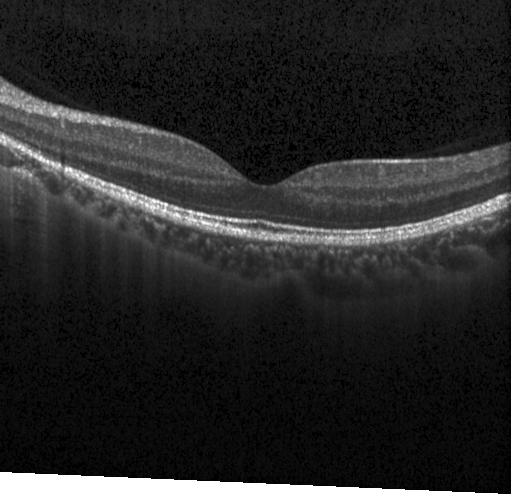 Diagnosis: no evidence of CNV, DME, or drusen.